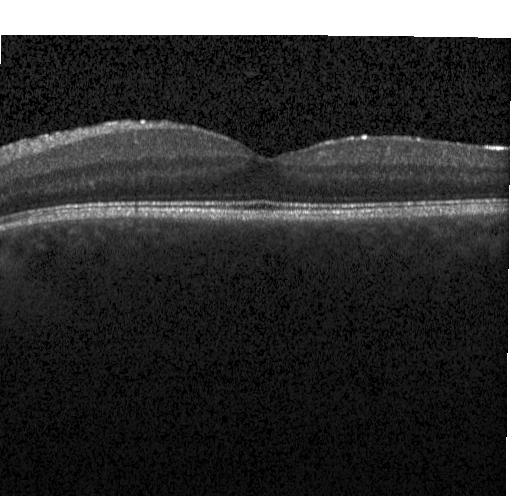 SD-OCT; through the macula; retinal OCT cross-section
OCT finding: no evidence of choroidal neovascularization, diabetic macular edema, or drusen.